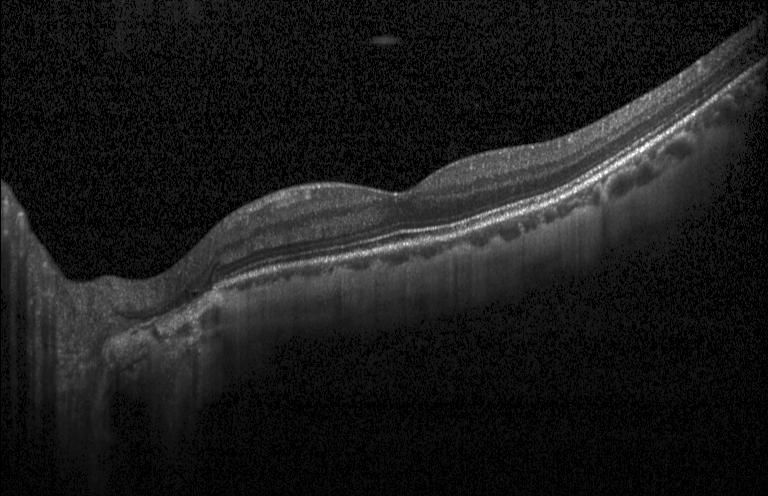
OCT B-scan.
Assessment: no CNV, DME, or drusen.